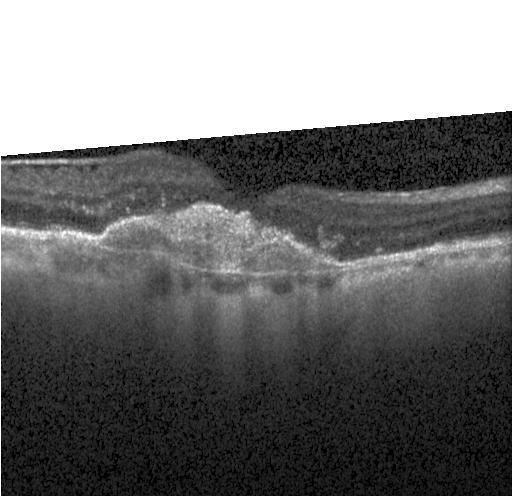

OCT line scan; through the macula — Impression: a choroidal neovascular membrane.